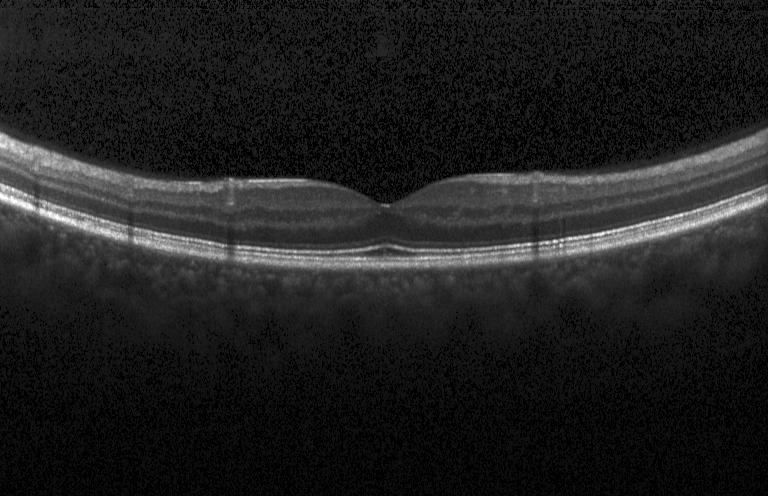
Macular scan · OCT B-scan.
Diagnosis: neither choroidal neovascularization, diabetic macular edema, nor drusen.